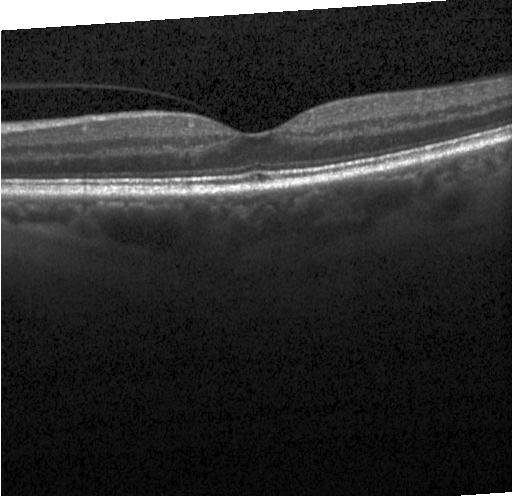 Dx: no choroidal neovascularization, diabetic macular edema, or drusen.